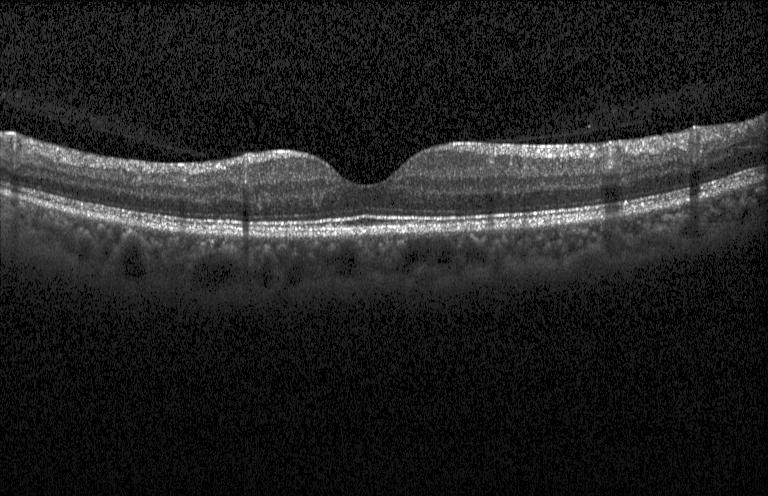 Retinal OCT B-scan · Heidelberg Spectralis
Finding: no CNV, DME, or drusen.